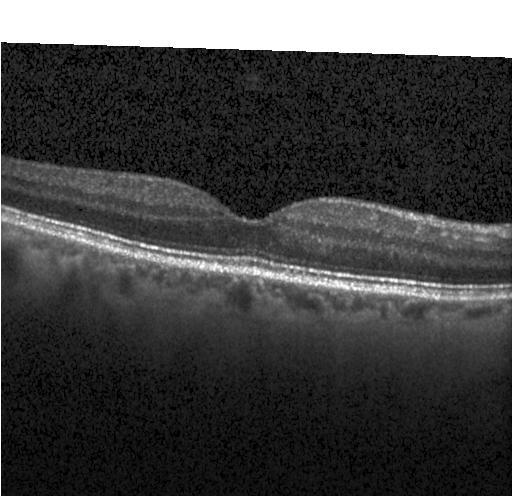 OCT finding: no choroidal neovascularization, no diabetic macular edema, and no drusen.